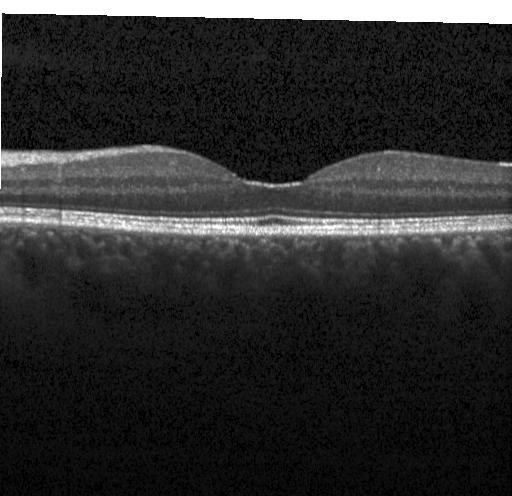

OCT finding: no choroidal neovascularization, diabetic macular edema, or drusen.